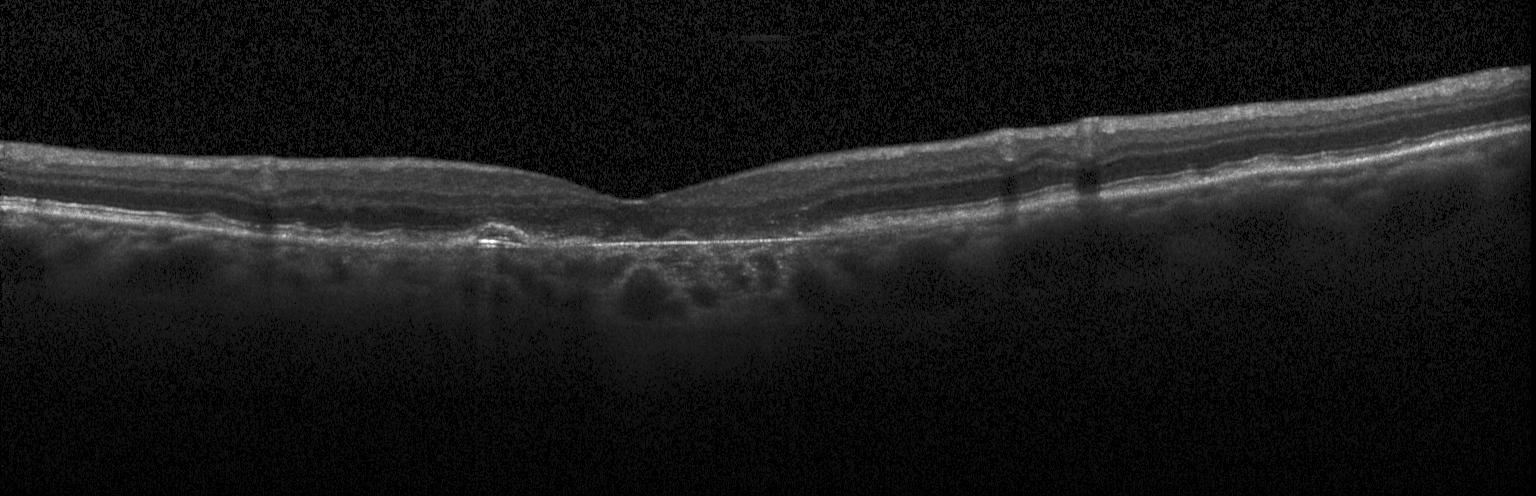 Optical coherence tomography scan — Finding: choroidal neovascularization (CNV).